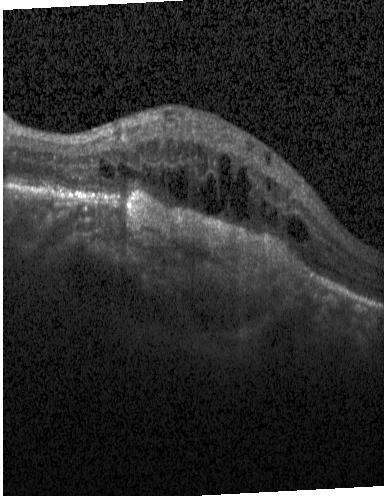
Fovea-centered, OCT B-scan. Finding: choroidal neovascularization (CNV).